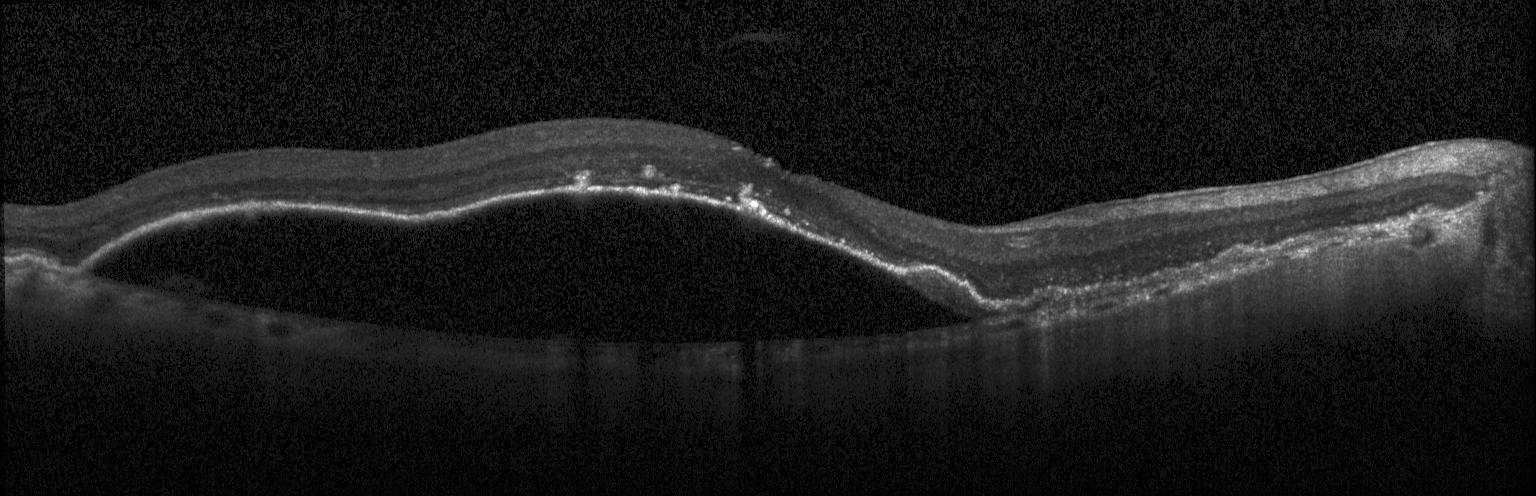

Spectral-domain optical coherence tomography · Heidelberg Spectralis OCT system · macular scan · retinal OCT B-scan. Diagnosis: choroidal neovascularization (CNV).